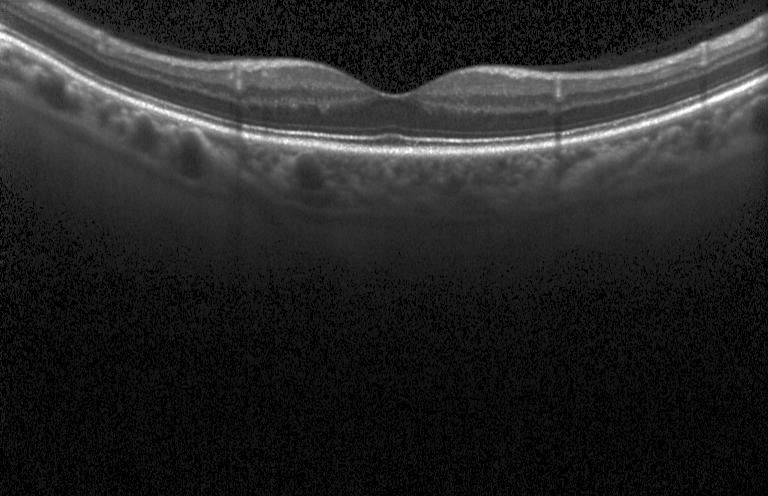

OCT B-scan; centered on the fovea.
The scan shows neither CNV, DME, nor drusen.